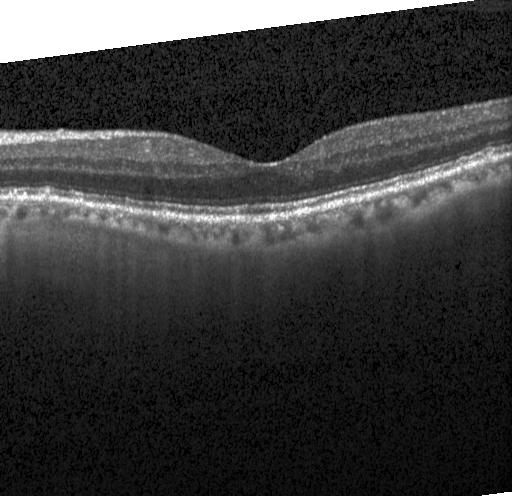 OCT B-scan; Heidelberg Spectralis OCT system. No choroidal neovascularization, diabetic macular edema, or drusen.